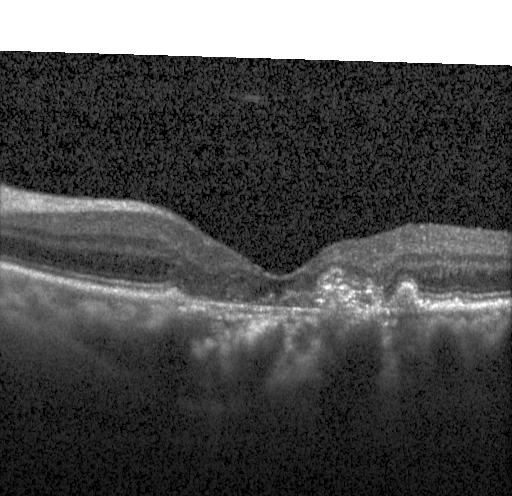 Instrument: Heidelberg Spectralis · optical coherence tomography scan
Finding: choroidal neovascularization.